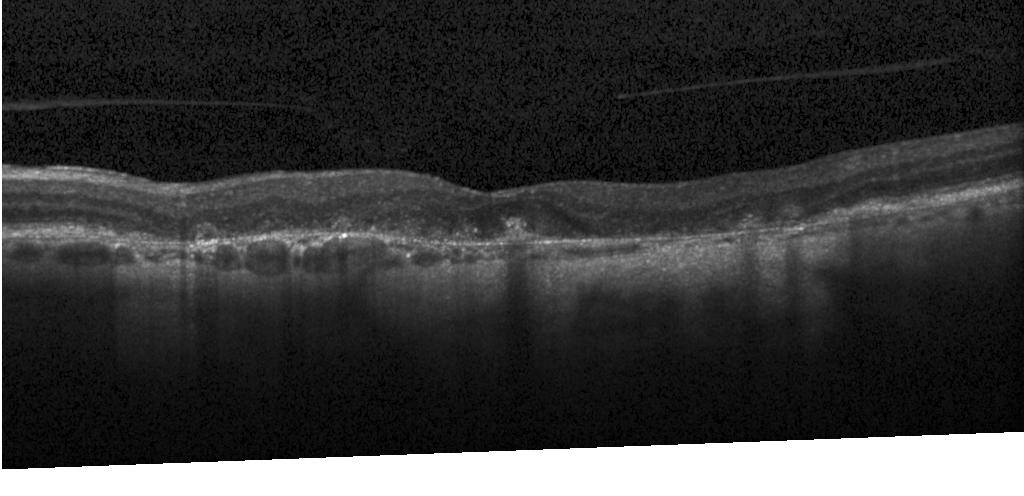

Impression: no evidence of CNV, DME, or drusen.